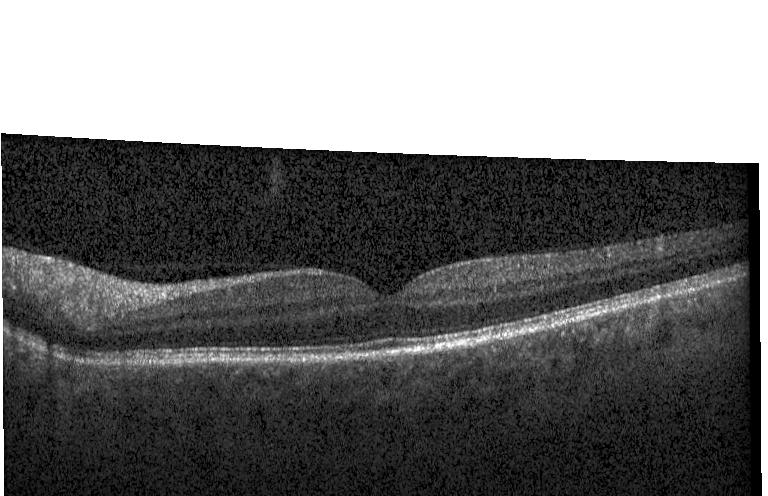
OCT line scan · SD-OCT.
OCT finding: neither CNV, DME, nor drusen.